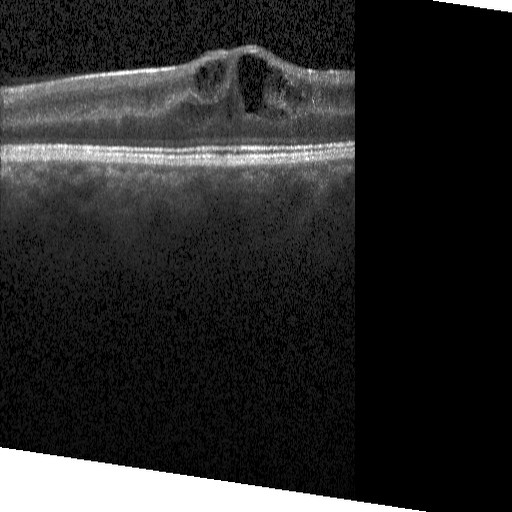 Macular OCT demonstrating DME.